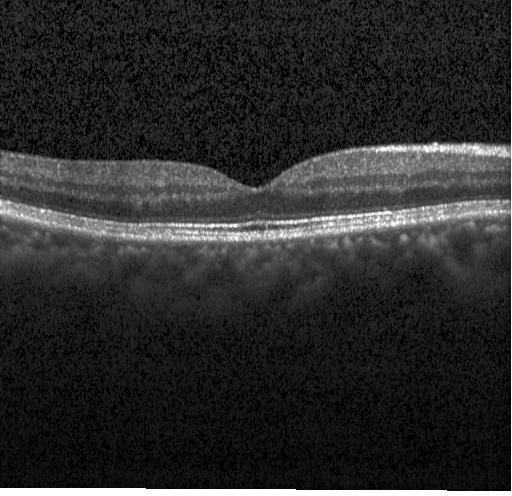
Heidelberg Spectralis OCT system; spectral-domain optical coherence tomography; OCT line scan; horizontal scan through the fovea — The scan shows no evidence of CNV, DME, or drusen.